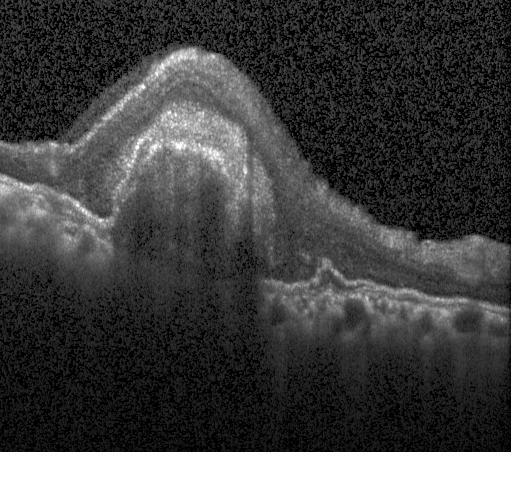

Macular scan; optical coherence tomography scan.
Finding: CNV.